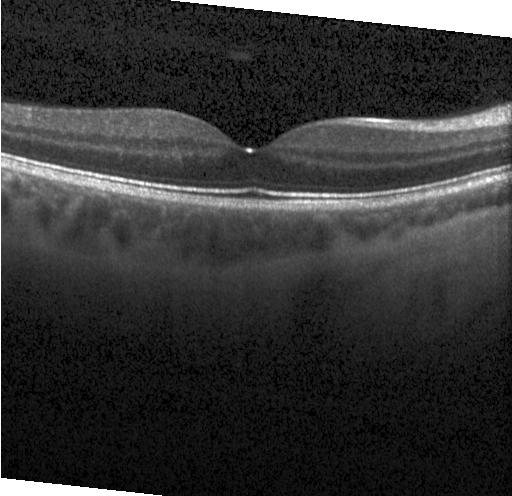 Acquired on a Heidelberg Spectralis, spectral-domain optical coherence tomography, optical coherence tomography B-scan
Diagnosis: no choroidal neovascularization, no diabetic macular edema, and no drusen.